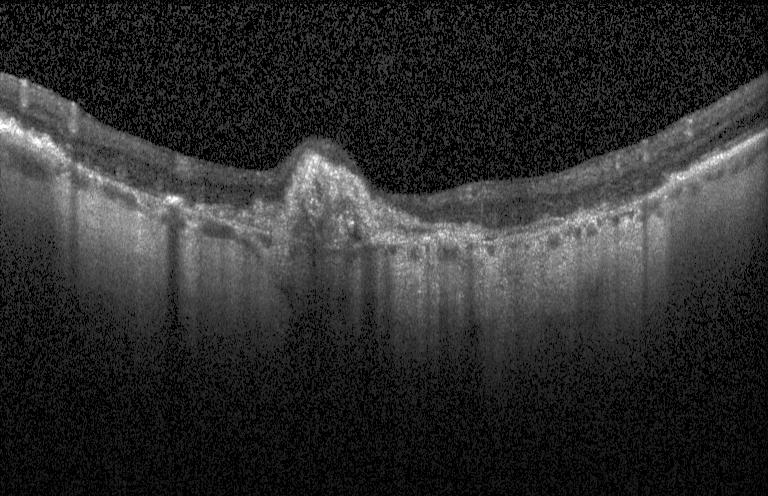

Fovea-centered · Heidelberg Spectralis · optical coherence tomography B-scan
This B-scan demonstrates choroidal neovascularization (CNV).